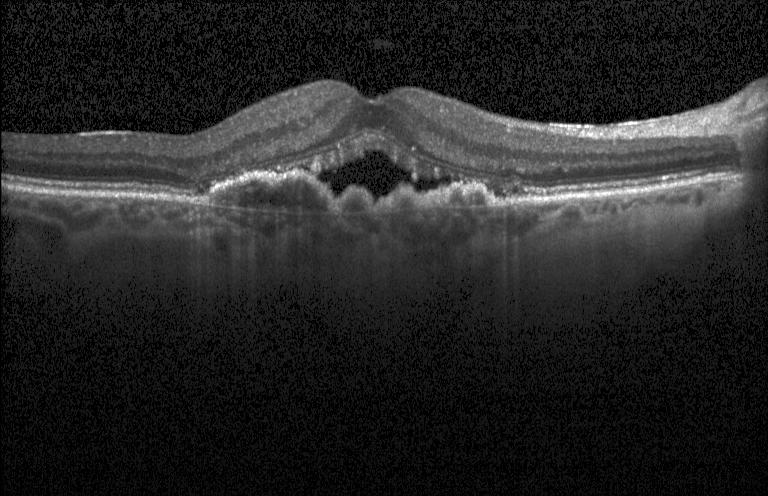 OCT finding: a choroidal neovascular membrane.